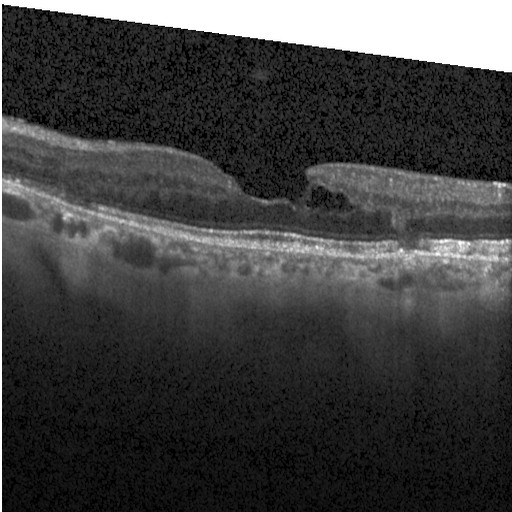 Retinal OCT cross-section showing DME.